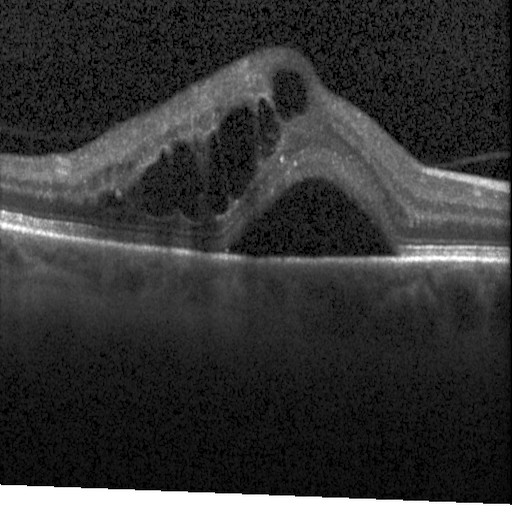

SD-OCT; Heidelberg Spectralis OCT system; retinal OCT cross-section; macular scan — Impression: diabetic macular edema.